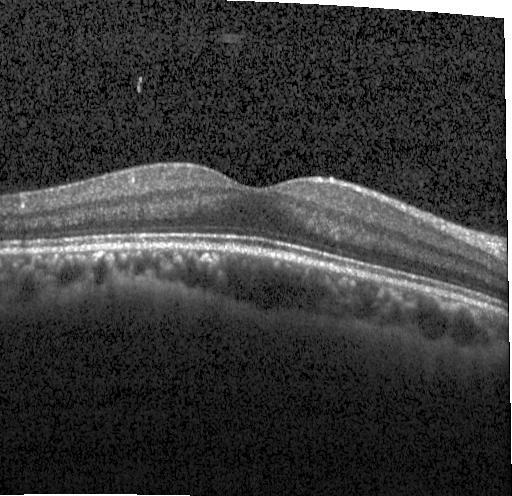

Impression: no CNV, DME, or drusen.